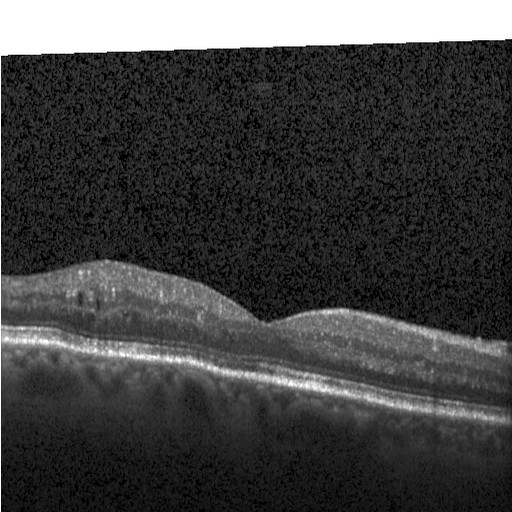

OCT line scan · SD-OCT · acquired on a Heidelberg Spectralis — Dx: DME.